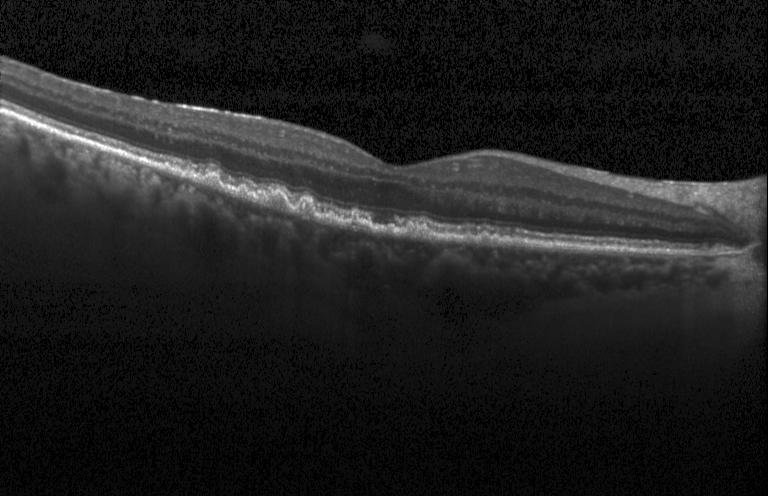 Fovea-centered; retinal OCT cross-section — Finding: sub-RPE drusenoid deposits.